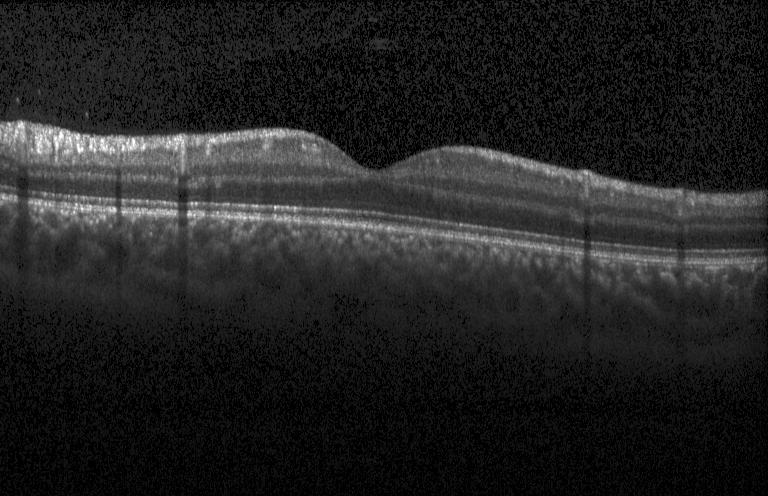

This B-scan demonstrates no choroidal neovascularization, no diabetic macular edema, and no drusen.